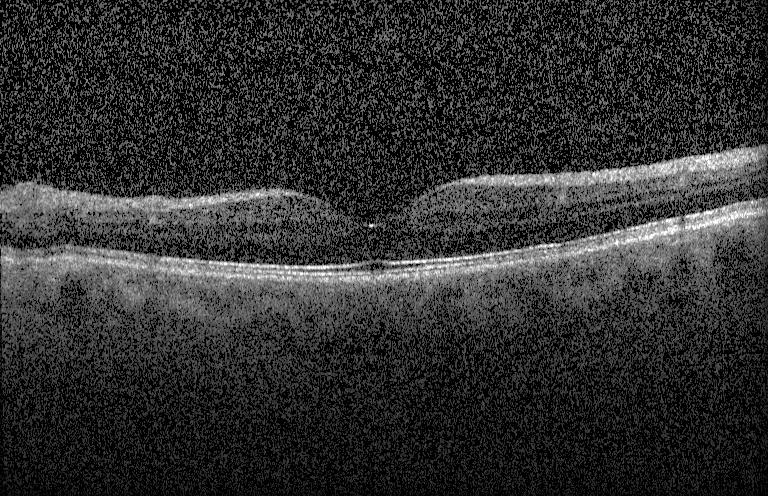 Retinal OCT cross-section. No CNV, no DME, and no drusen.